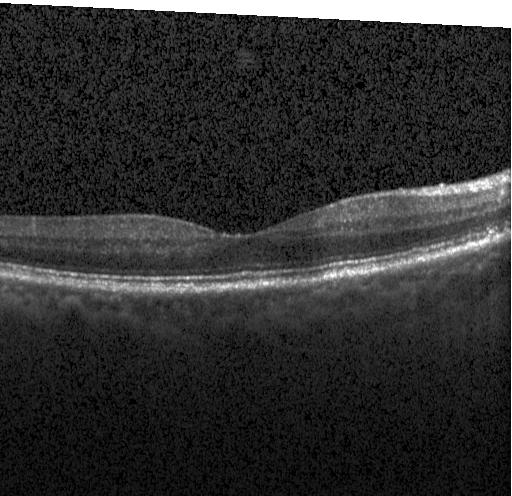 Horizontal scan through the fovea; Heidelberg Spectralis; optical coherence tomography scan.
Diagnosis: no choroidal neovascularization, no diabetic macular edema, and no drusen.